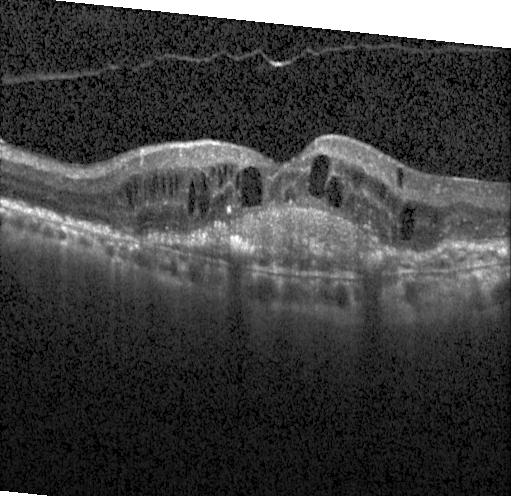

OCT line scan; spectral-domain OCT — Finding: choroidal neovascularization.